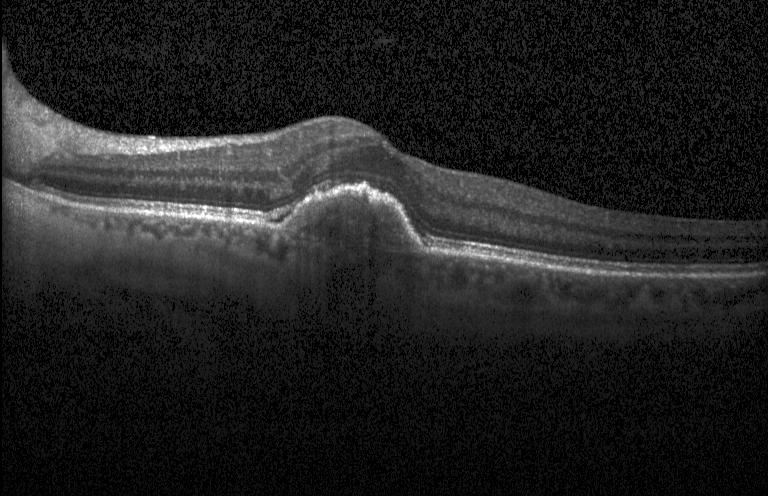 Optical coherence tomography B-scan
Impression: choroidal neovascularization (CNV).